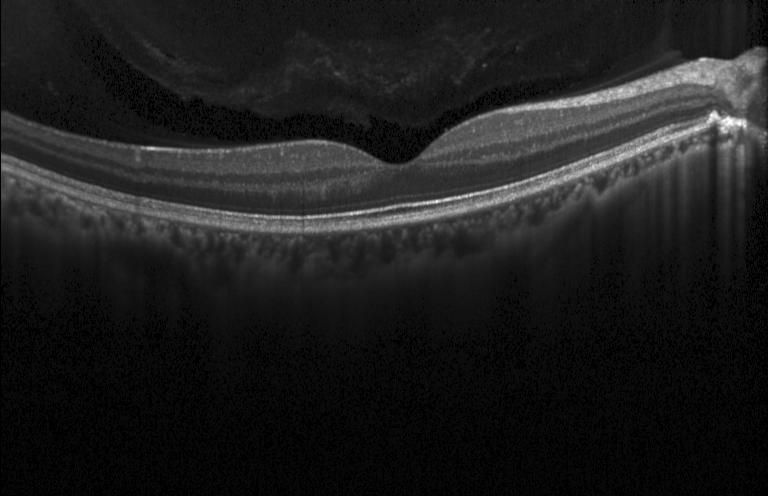

OCT finding: no evidence of choroidal neovascularization, diabetic macular edema, or drusen.